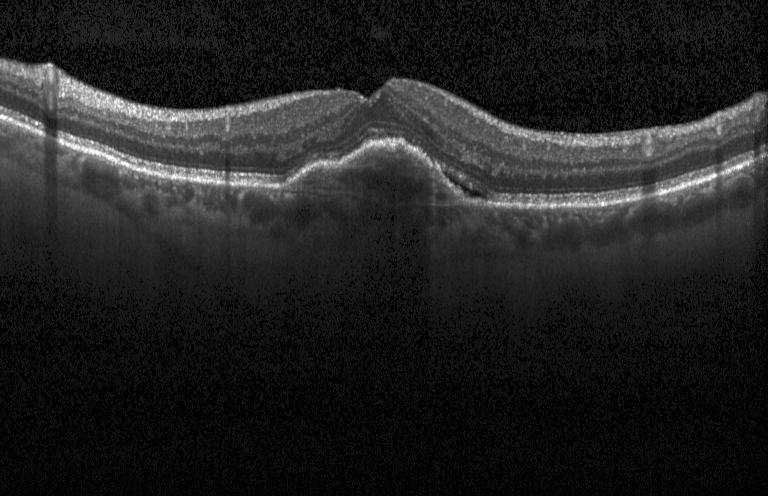
Spectral-domain OCT B-scan: CNV.